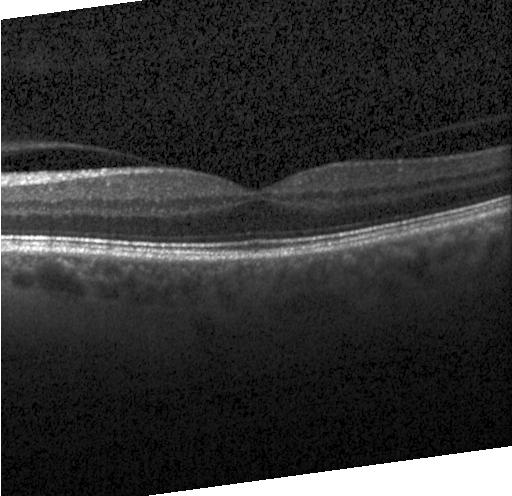 Fovea-centered. Heidelberg Spectralis. OCT line scan.
Diagnosis: no evidence of CNV, DME, or drusen.